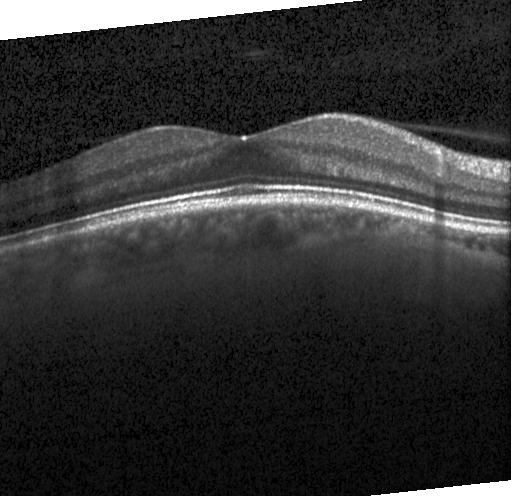 Impression: no CNV, DME, or drusen.